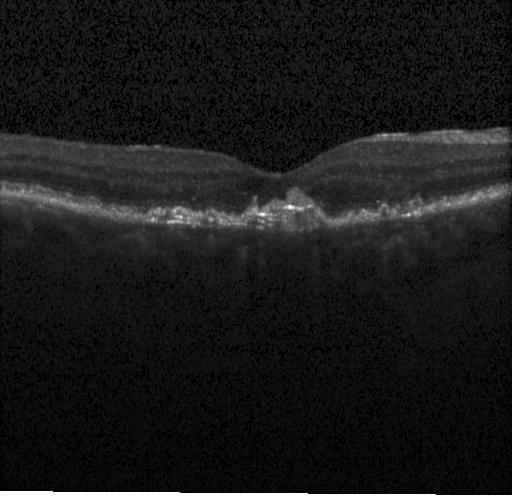
This B-scan demonstrates choroidal neovascularization (CNV).